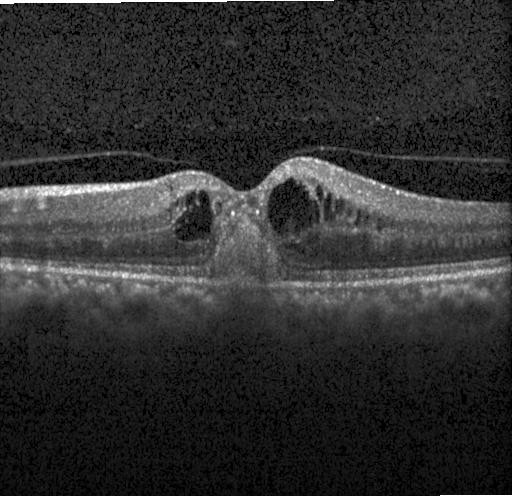

Finding: choroidal neovascularization.